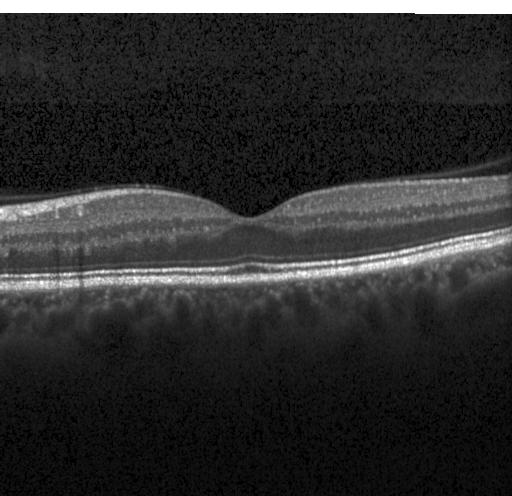

Heidelberg Spectralis OCT system, optical coherence tomography scan — Assessment: neither CNV, DME, nor drusen.